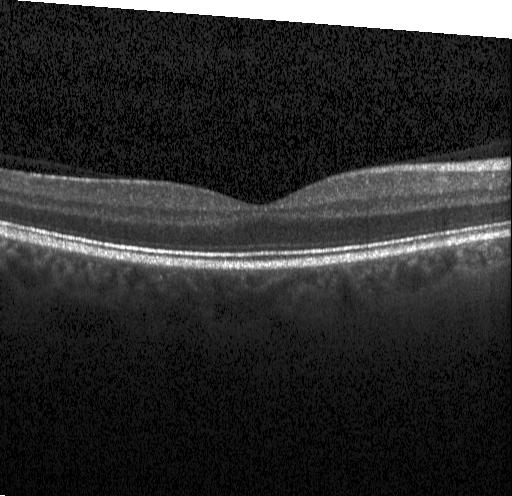 SD-OCT. Heidelberg Spectralis. Optical coherence tomography scan.
Finding: no evidence of choroidal neovascularization, diabetic macular edema, or drusen.